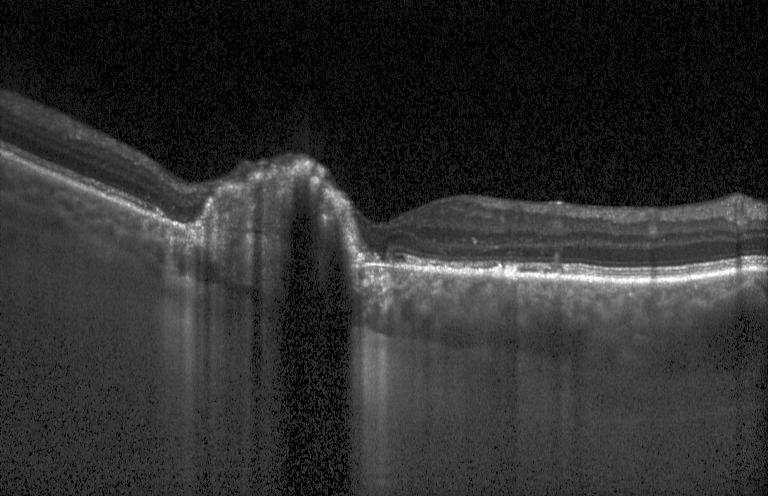 Optical coherence tomography B-scan · spectral-domain OCT · acquired on a Heidelberg Spectralis — Finding: choroidal neovascularization (CNV).